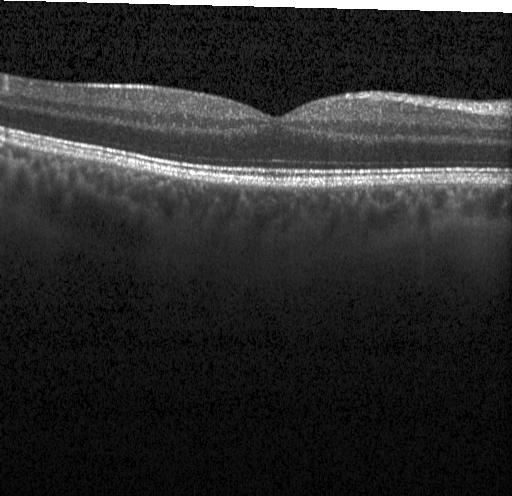

Optical coherence tomography B-scan · instrument: Heidelberg Spectralis · through the macula · spectral-domain OCT — Dx: no choroidal neovascularization, no diabetic macular edema, and no drusen.